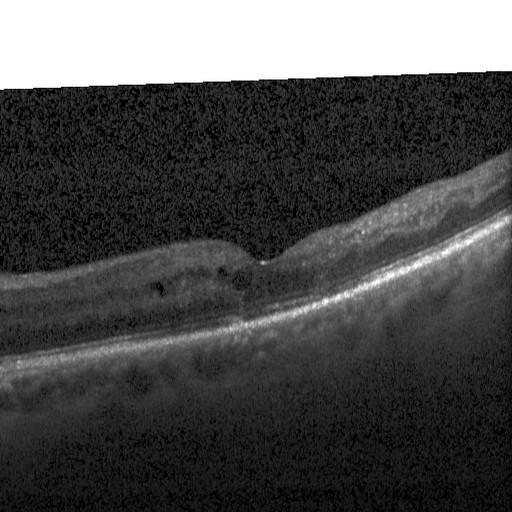 SD-OCT; retinal OCT cross-section; centered on the fovea; instrument: Heidelberg Spectralis.
The scan shows diabetic macular edema (DME).